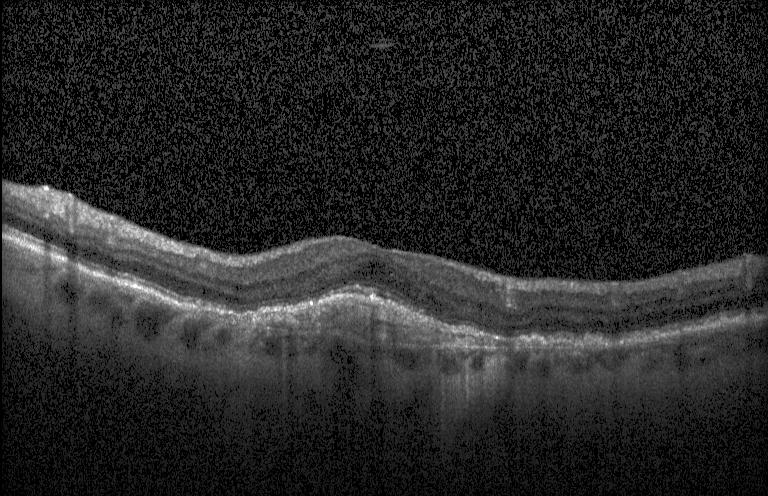
SD-OCT. Retinal OCT B-scan. Acquired on a Heidelberg Spectralis. Impression: a choroidal neovascular membrane.